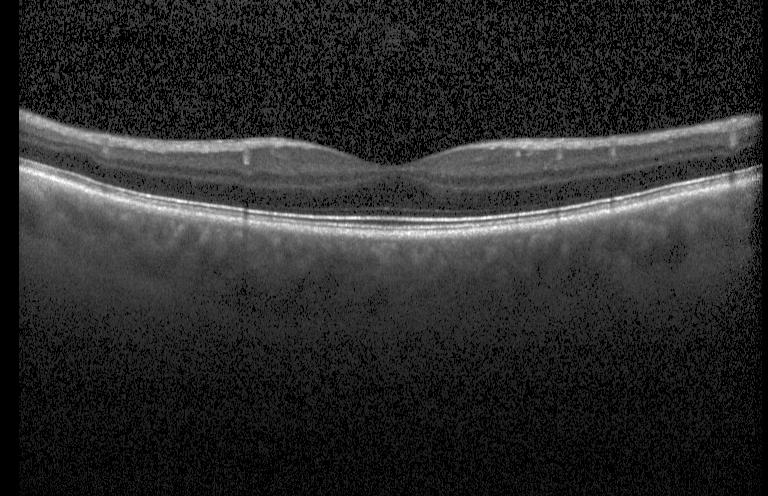 This B-scan demonstrates no choroidal neovascularization, no diabetic macular edema, and no drusen.